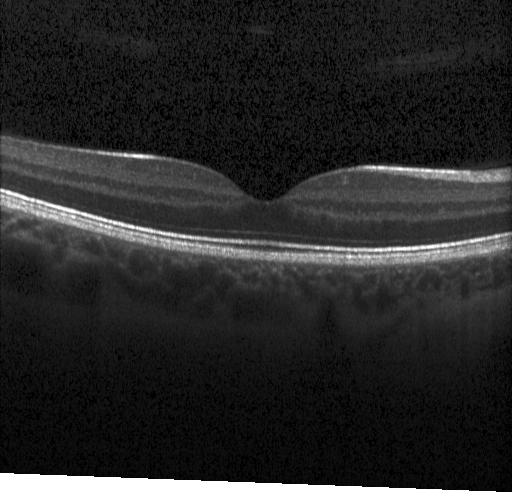 Retinal OCT B-scan; spectral-domain OCT
No CNV, no DME, and no drusen.